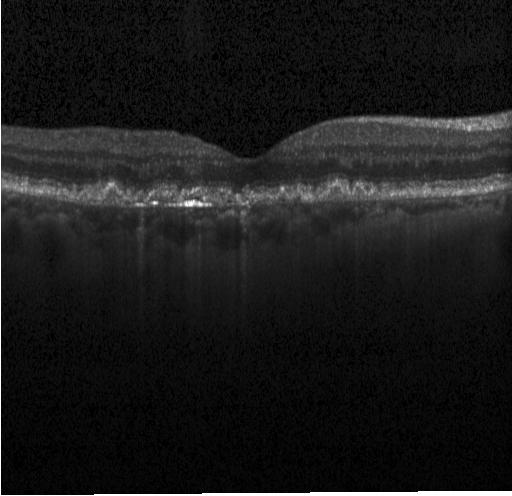 Impression: CNV.